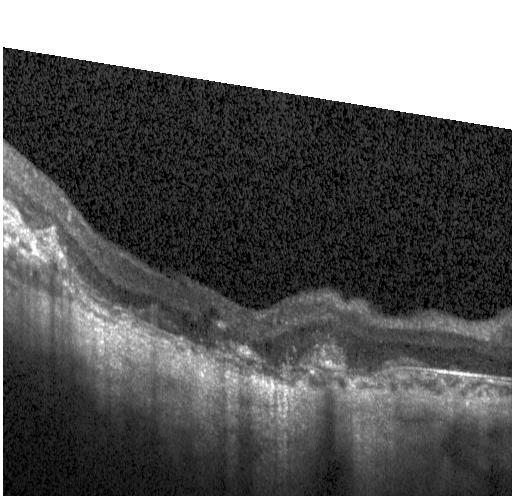 The scan shows choroidal neovascularization.